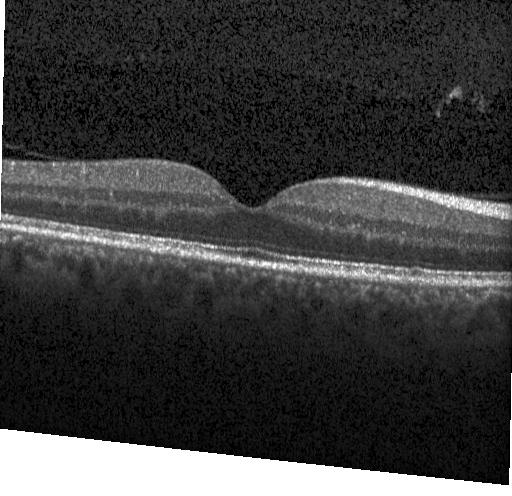 Instrument: Heidelberg Spectralis; optical coherence tomography scan; macular scan; spectral-domain optical coherence tomography
Dx: no evidence of CNV, DME, or drusen.